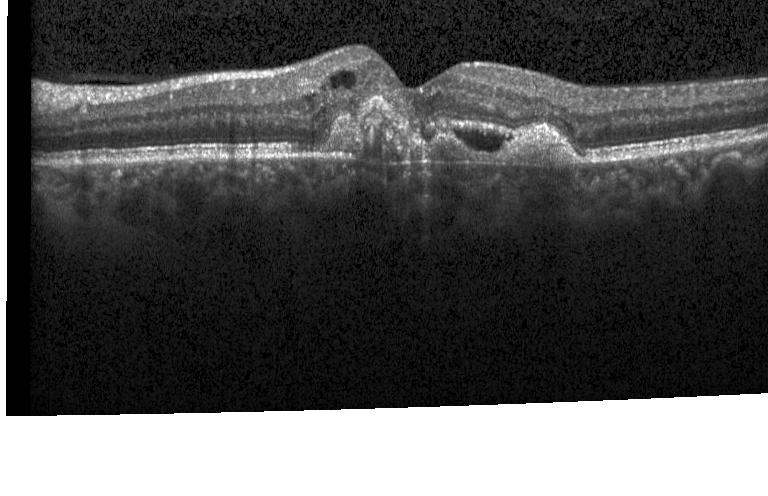 OCT finding: a choroidal neovascular membrane.